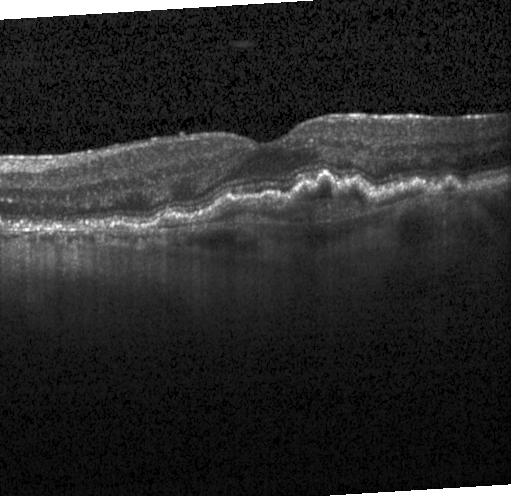
Optical coherence tomography B-scan, spectral-domain OCT.
Impression: a choroidal neovascular membrane.